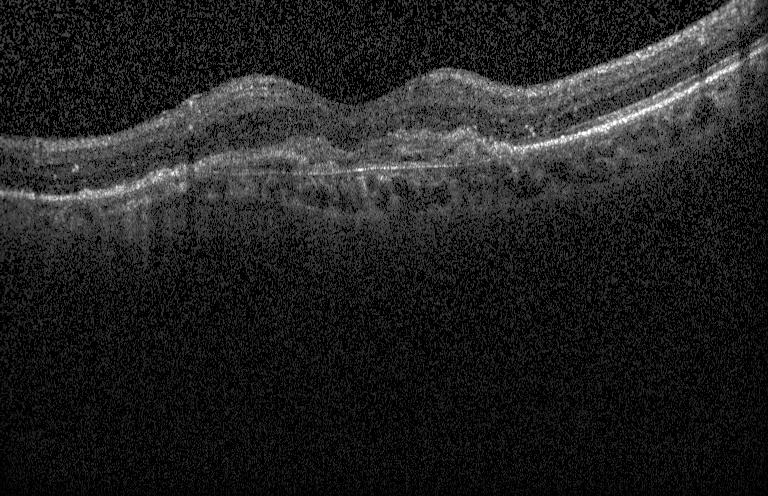

Macular OCT: a choroidal neovascular membrane.